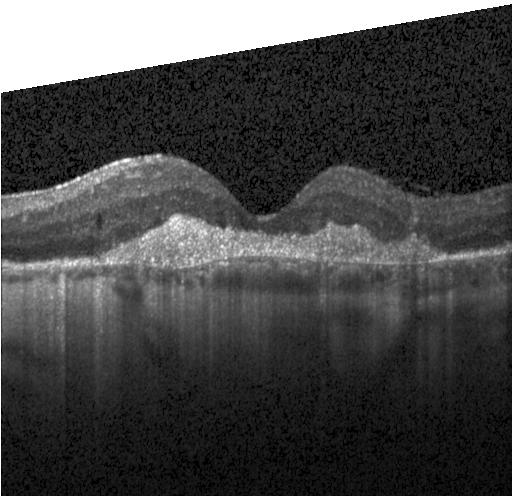
Horizontal scan through the fovea. OCT B-scan. Acquired on a Heidelberg Spectralis. Spectral-domain optical coherence tomography.
Impression: CNV.